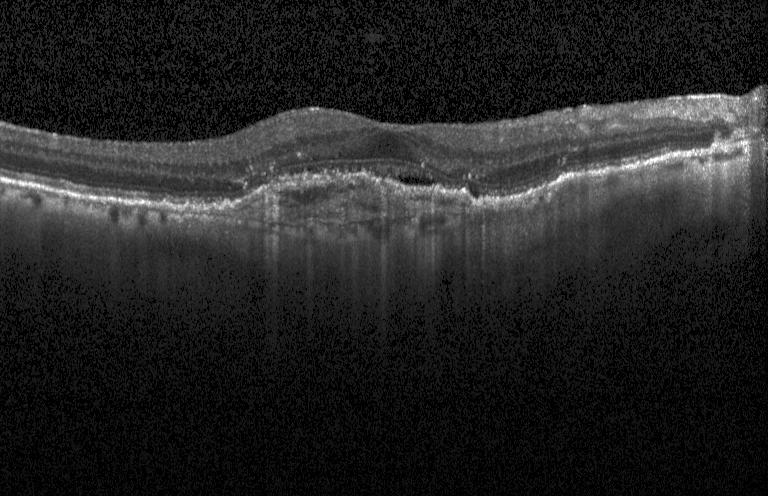 Retinal OCT B-scan
A choroidal neovascular membrane.